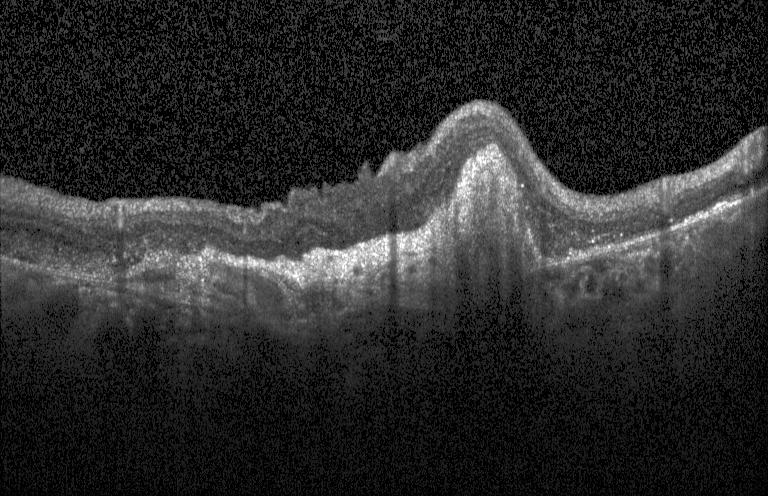

Finding: choroidal neovascularization.